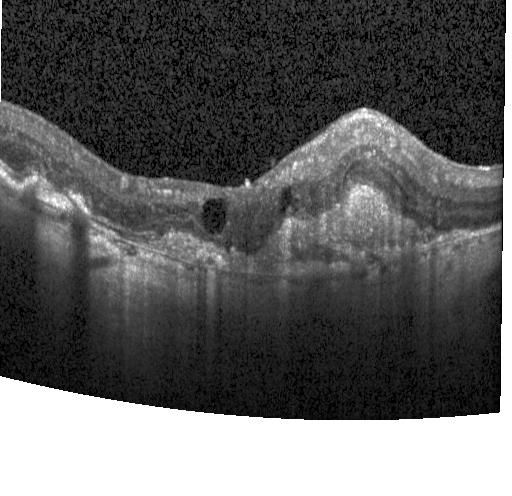 Instrument: Heidelberg Spectralis · OCT B-scan · fovea-centered. The scan shows choroidal neovascularization (CNV).